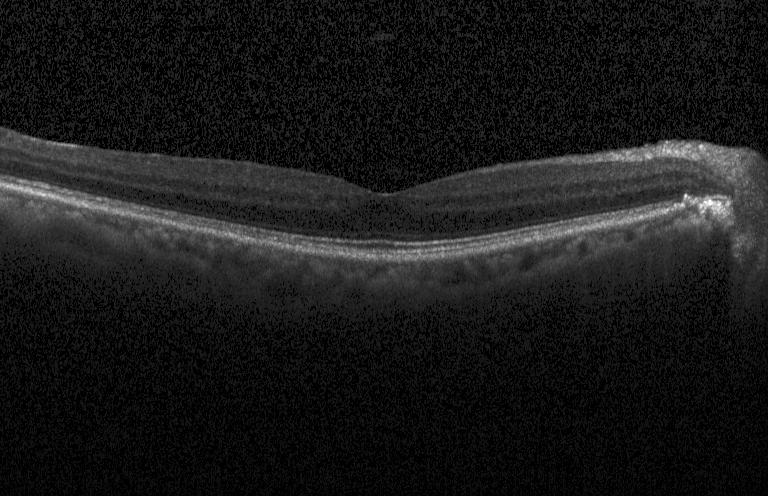
Finding: neither CNV, DME, nor drusen.